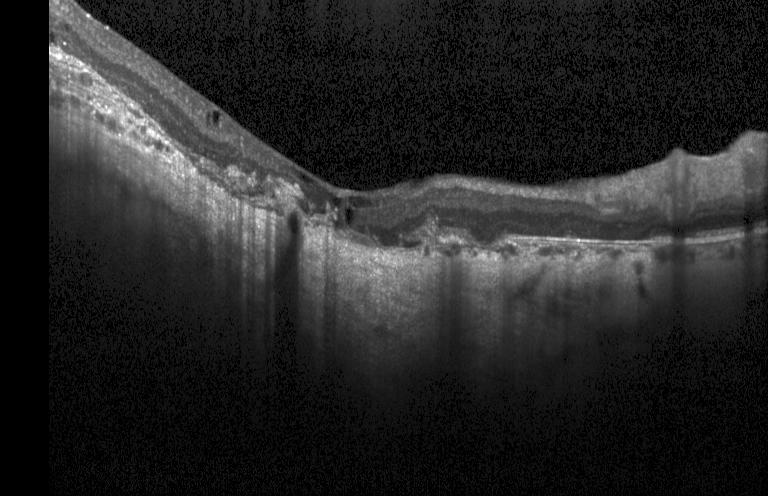

OCT finding: CNV.